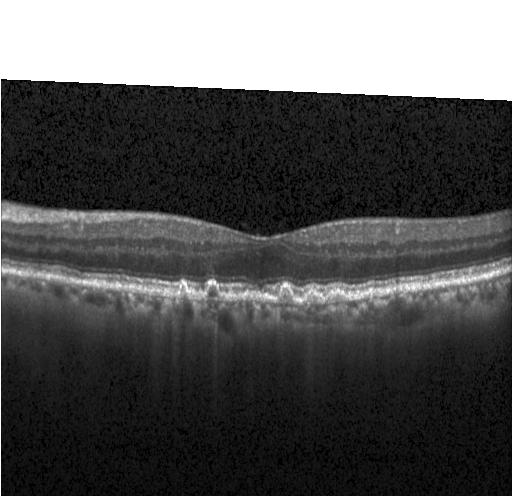 Optical coherence tomography B-scan. Heidelberg Spectralis. Macular scan — This B-scan demonstrates multiple drusen.